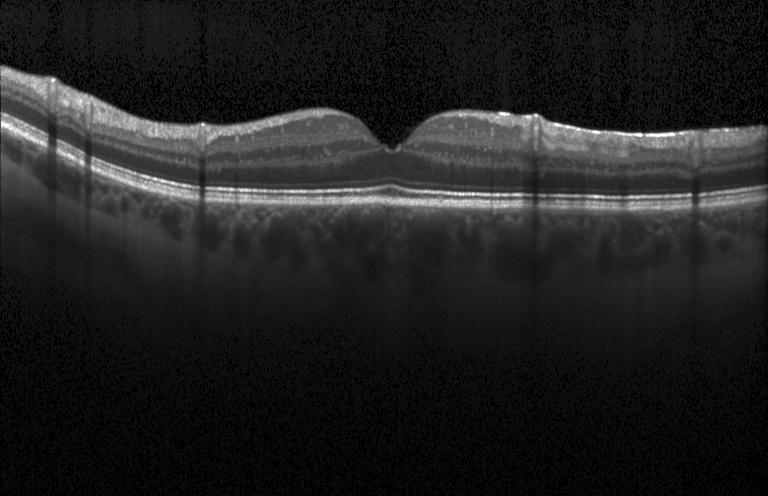

Finding: no choroidal neovascularization, no diabetic macular edema, and no drusen.